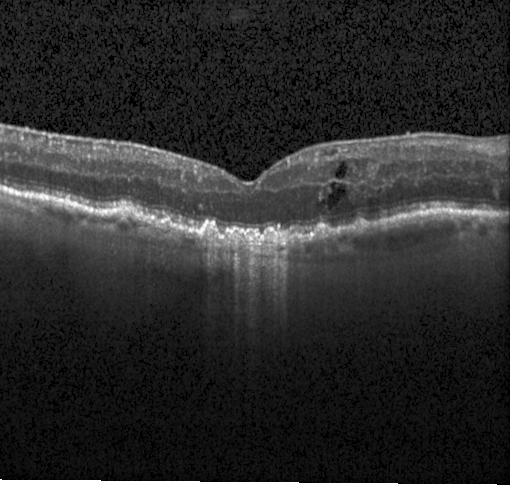

Spectral-domain optical coherence tomography. Horizontal scan through the fovea. Heidelberg Spectralis OCT system. Optical coherence tomography scan. Impression: choroidal neovascularization (CNV).